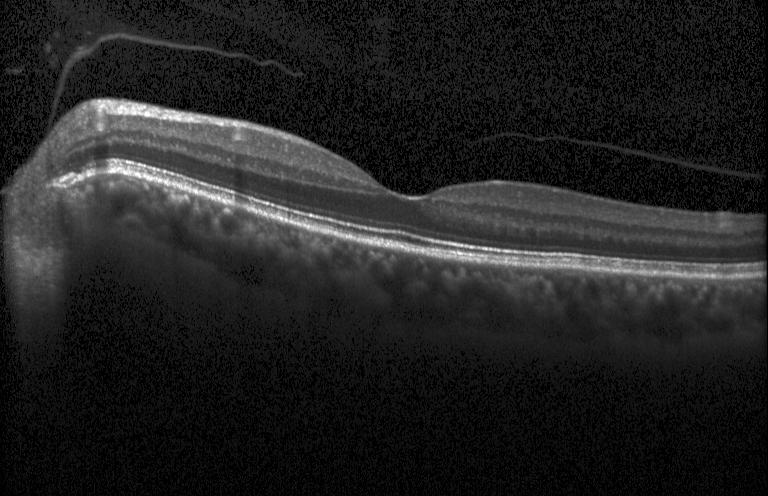 Impression: no evidence of choroidal neovascularization, diabetic macular edema, or drusen.